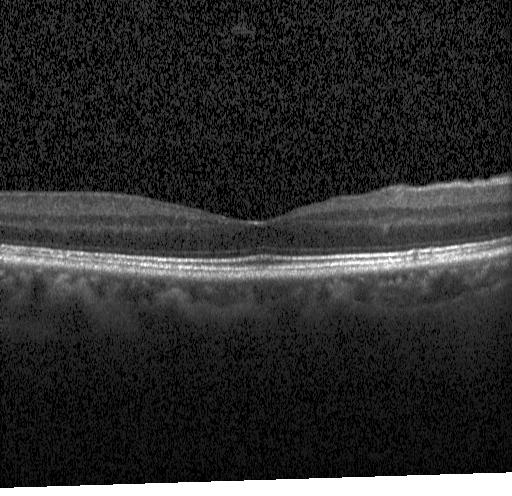 Spectral-domain optical coherence tomography, horizontal scan through the fovea, Heidelberg Spectralis, OCT line scan.
Dx: no choroidal neovascularization, no diabetic macular edema, and no drusen.